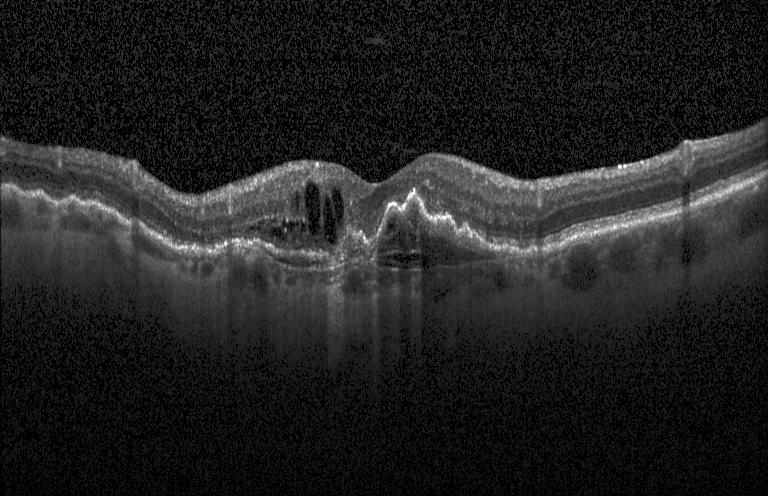
Spectral-domain OCT; Heidelberg Spectralis; retinal OCT B-scan.
Impression: choroidal neovascularization.